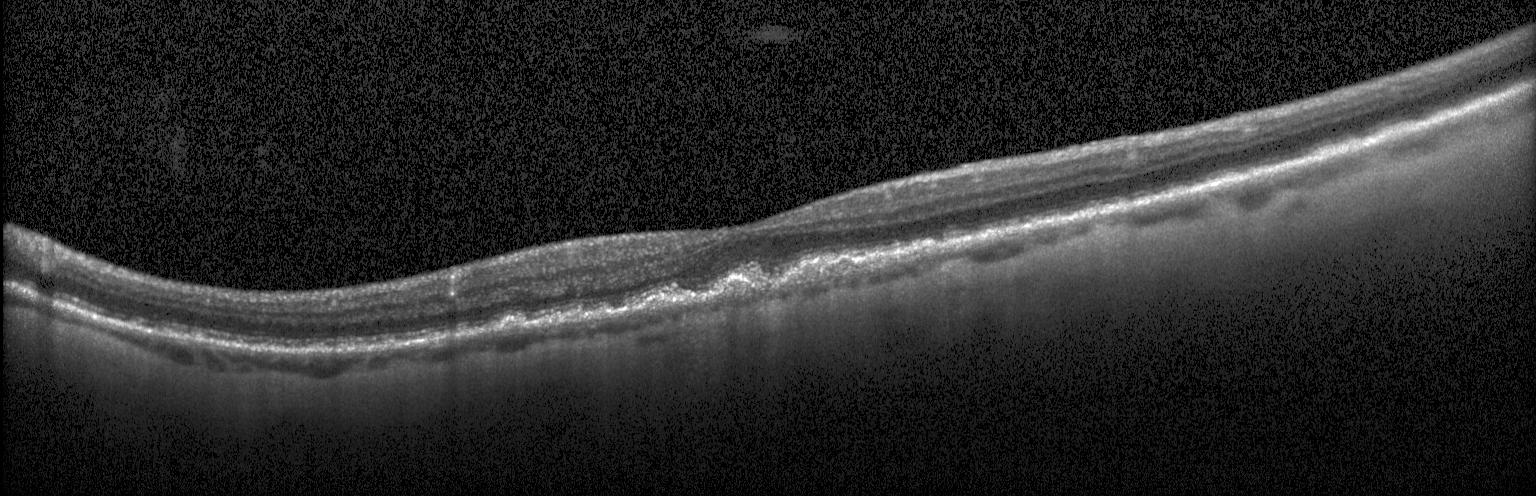 Finding: sub-RPE drusenoid deposits.